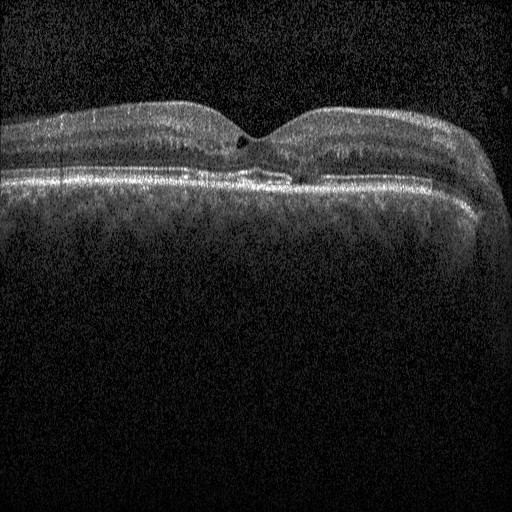 Macular OCT: DME.